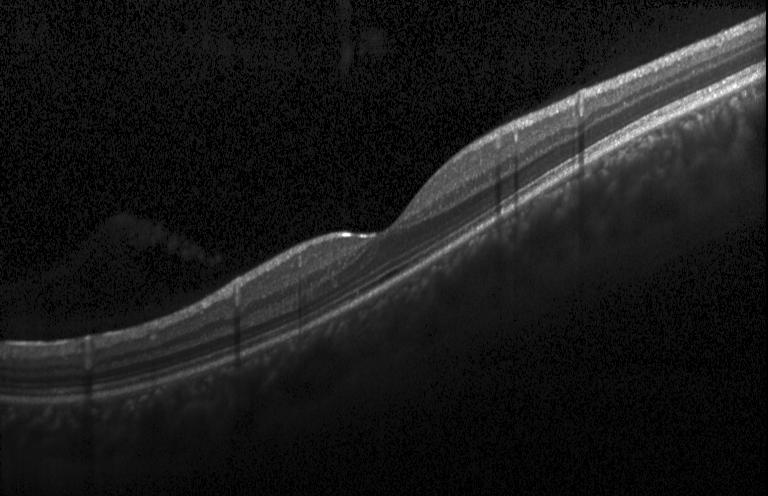
OCT B-scan. Diagnosis: neither choroidal neovascularization, diabetic macular edema, nor drusen.